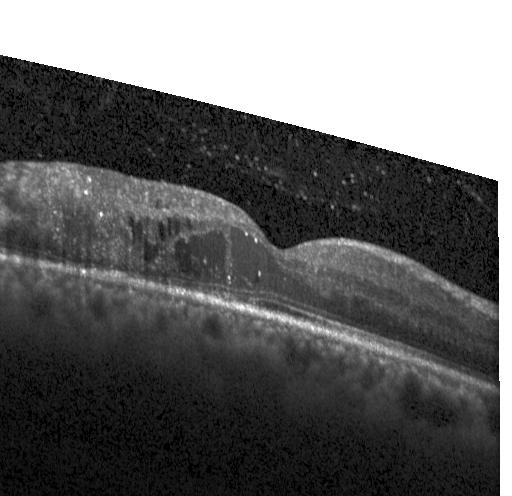
Spectral-domain OCT · Heidelberg Spectralis OCT system · OCT line scan · fovea-centered. The scan shows diabetic macular edema (DME).